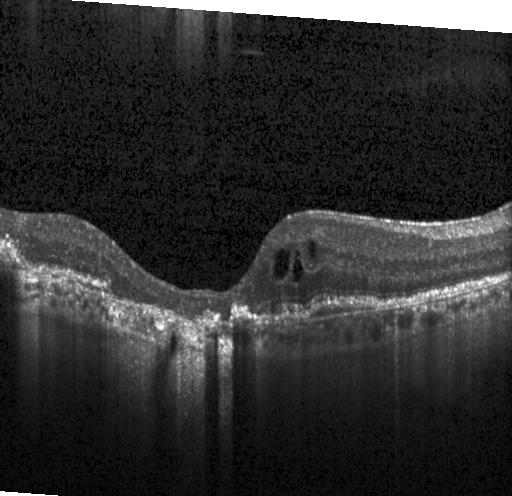

Assessment: a choroidal neovascular membrane.